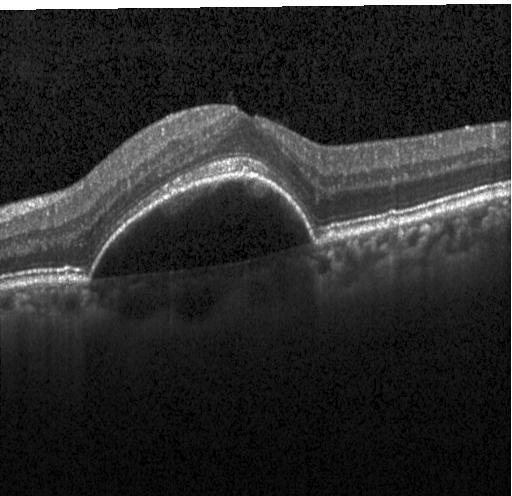 A choroidal neovascular membrane.